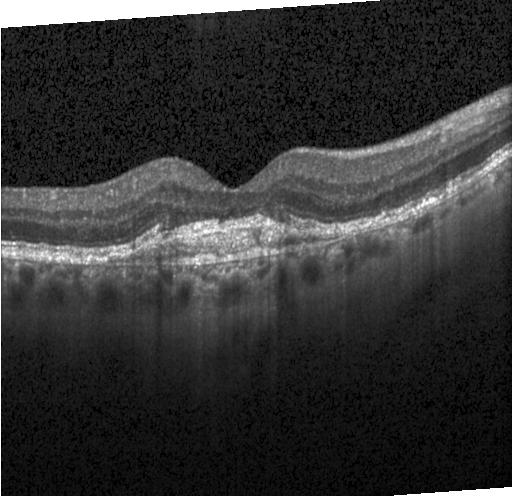 Horizontal scan through the fovea; Heidelberg Spectralis; OCT B-scan; spectral-domain OCT
Impression: choroidal neovascularization.